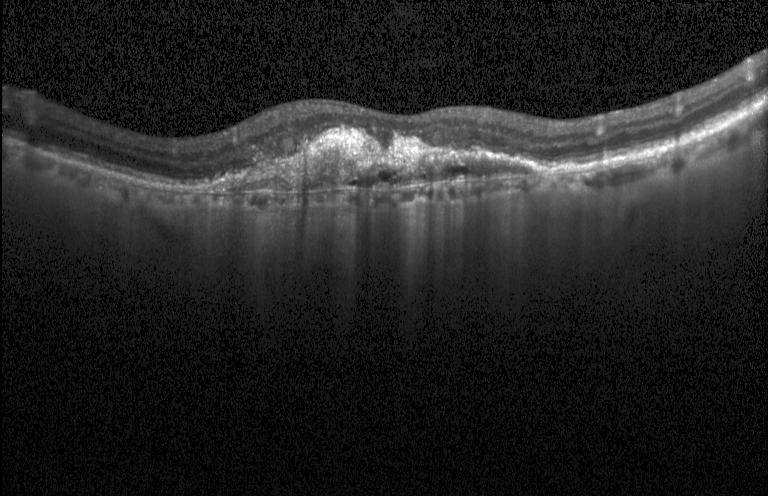 Optical coherence tomography B-scan. SD-OCT. Macular scan.
OCT finding: a choroidal neovascular membrane.